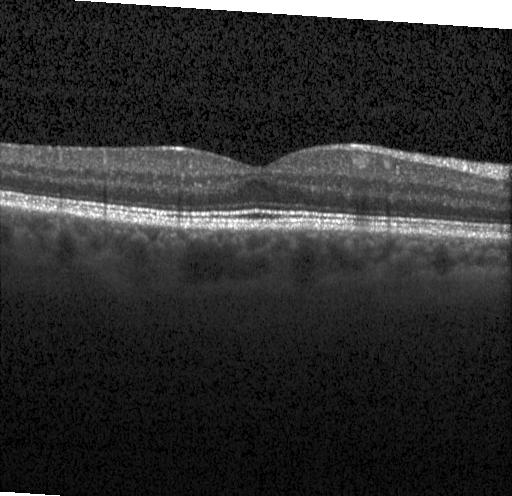 Heidelberg Spectralis, optical coherence tomography B-scan, fovea-centered. Macular OCT: no choroidal neovascularization, no diabetic macular edema, and no drusen.